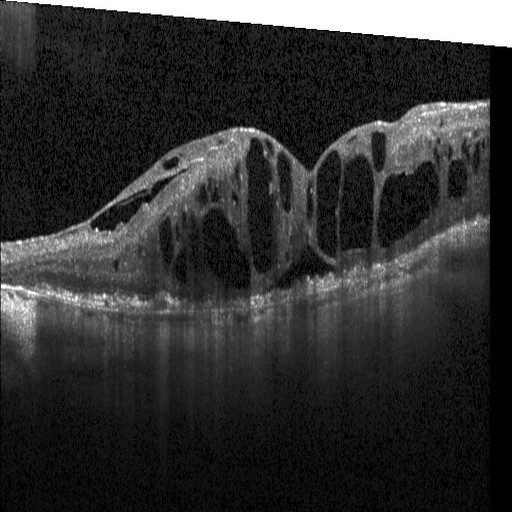

Retinal OCT B-scan — The scan shows diabetic macular edema.